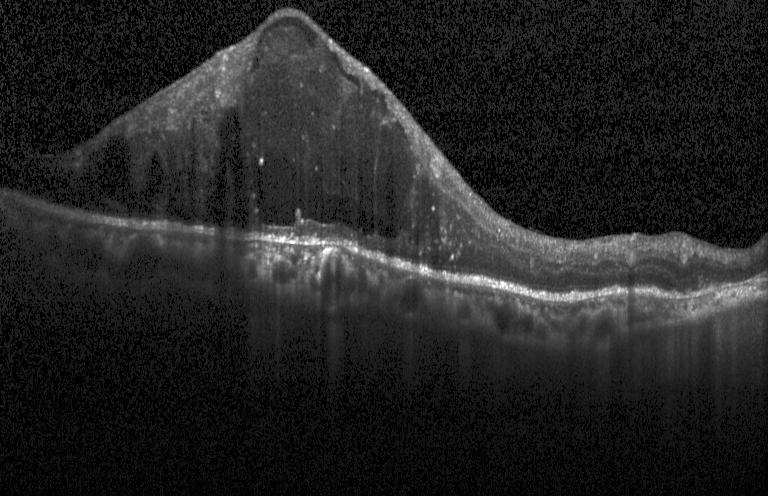 Retinal OCT B-scan, spectral-domain optical coherence tomography. Diagnosis: diabetic macular edema.